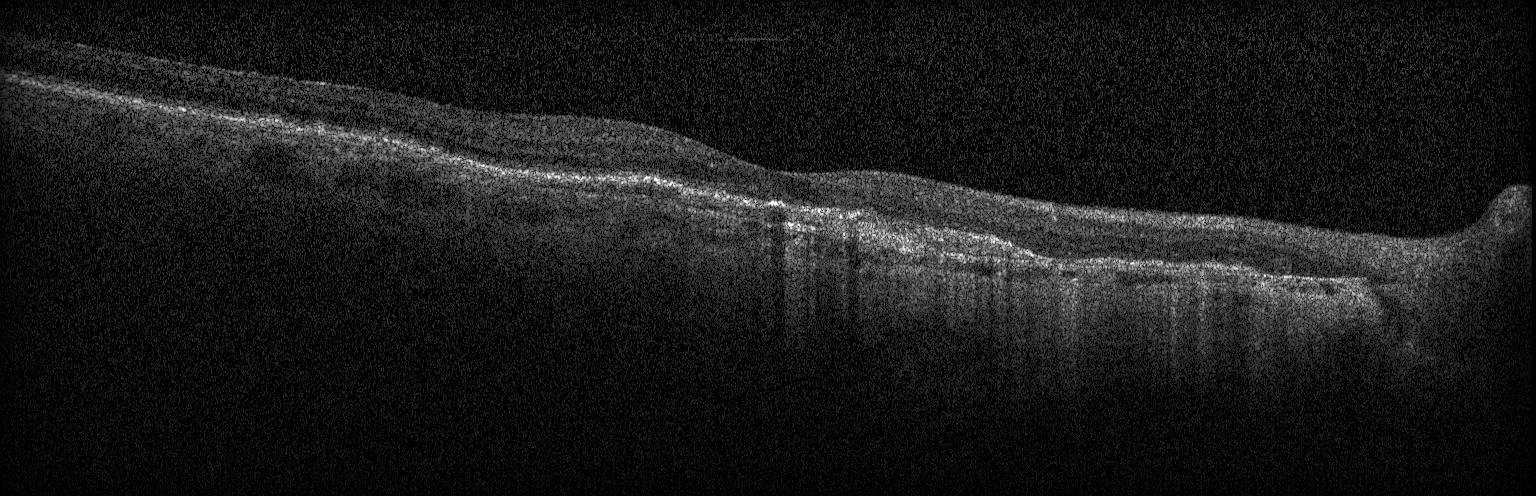

Heidelberg Spectralis; retinal OCT cross-section; through the macula; spectral-domain optical coherence tomography — Macular OCT: choroidal neovascularization (CNV).